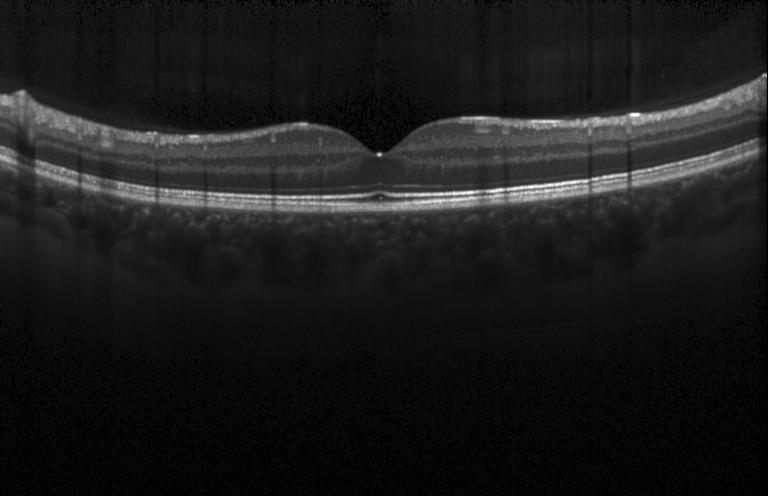
Assessment: neither CNV, DME, nor drusen.